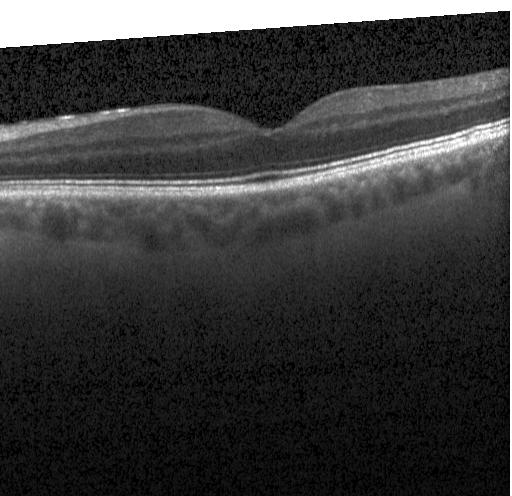 Optical coherence tomography scan — Diagnosis: no evidence of choroidal neovascularization, diabetic macular edema, or drusen.